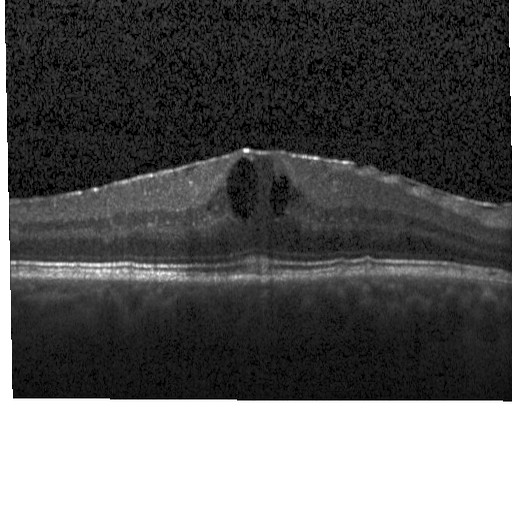 Diagnosis: diabetic macular edema.